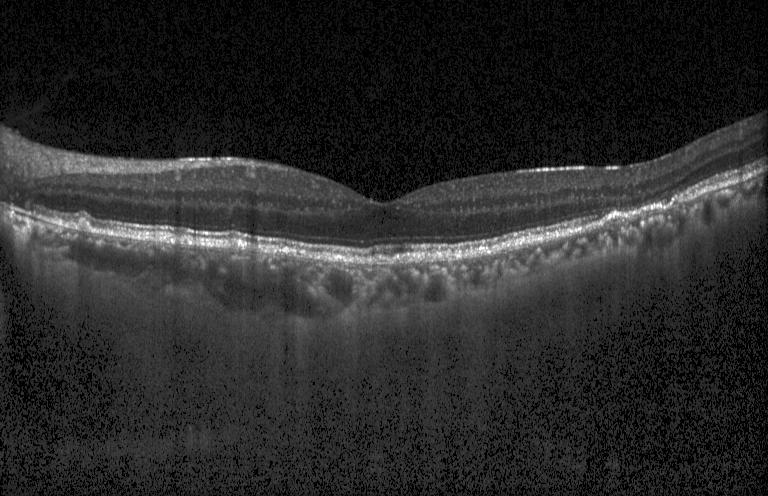

Dx: drusen.